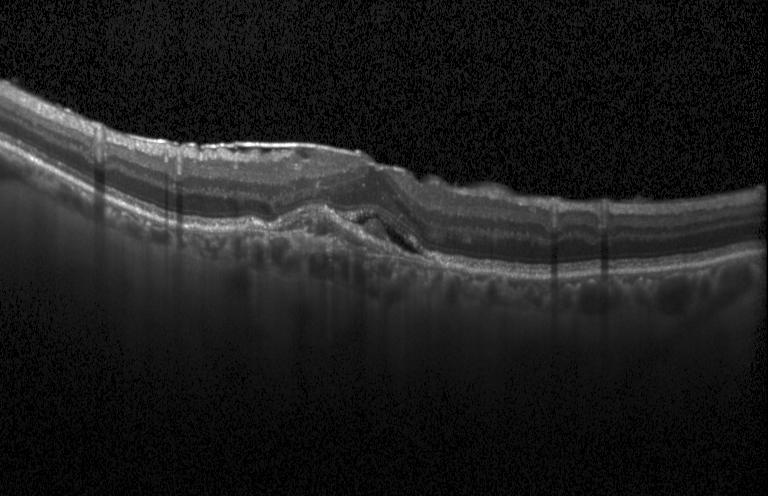

OCT scan showing CNV.